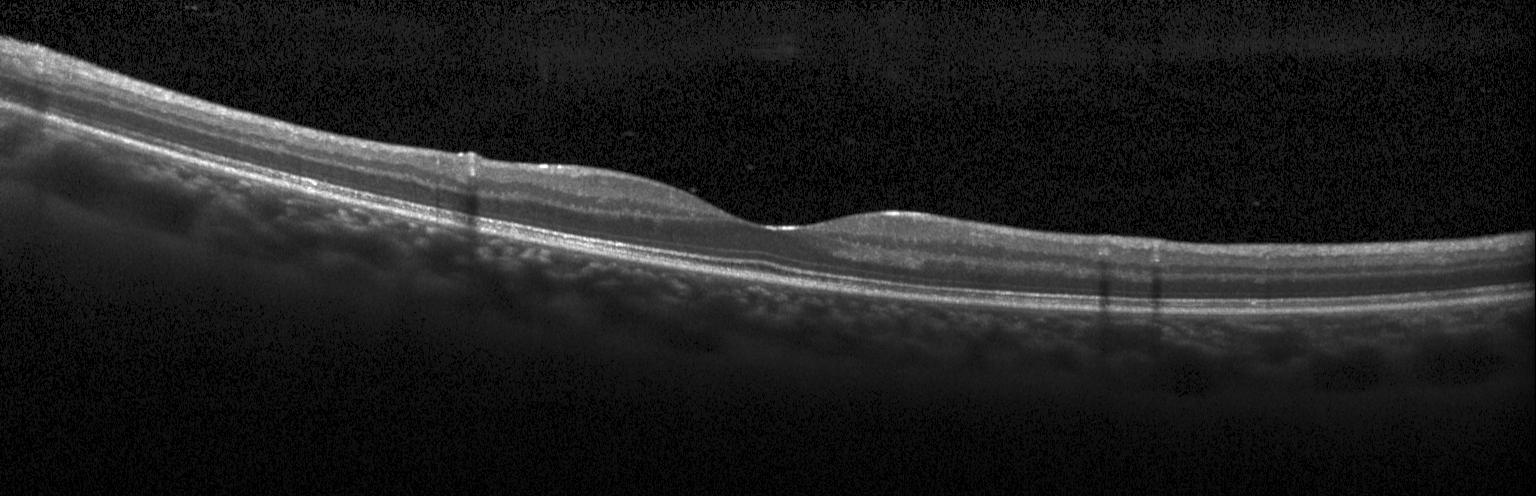
OCT finding: neither CNV, DME, nor drusen.